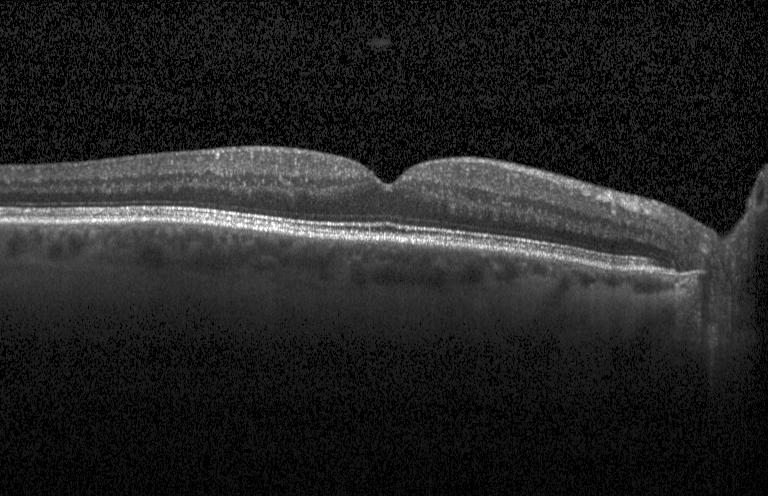 Retinal OCT cross-section · Heidelberg Spectralis OCT system — Macular OCT: no choroidal neovascularization, diabetic macular edema, or drusen.